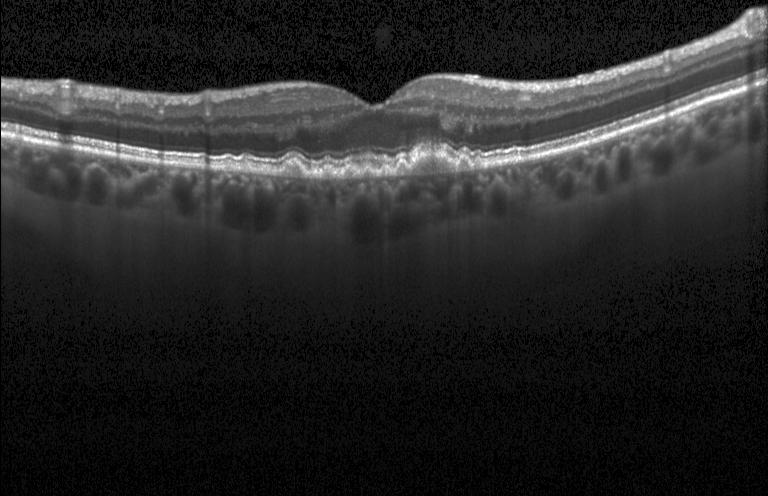

SD-OCT · macular scan · optical coherence tomography B-scan.
Assessment: drusen.